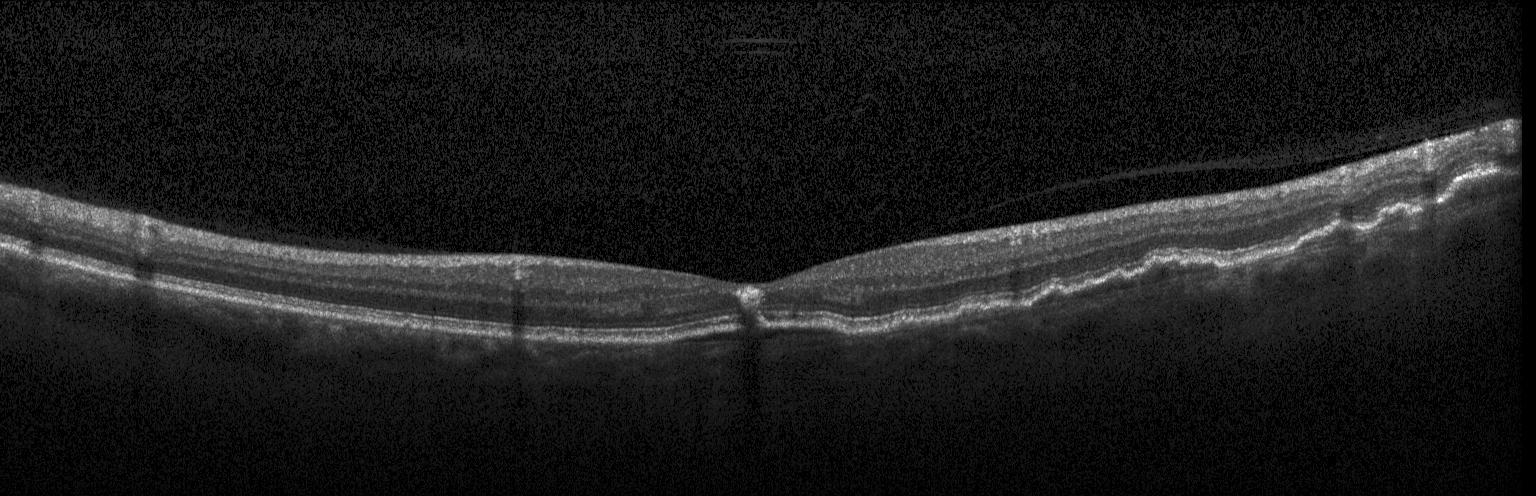

Horizontal scan through the fovea; optical coherence tomography scan; instrument: Heidelberg Spectralis
A choroidal neovascular membrane.